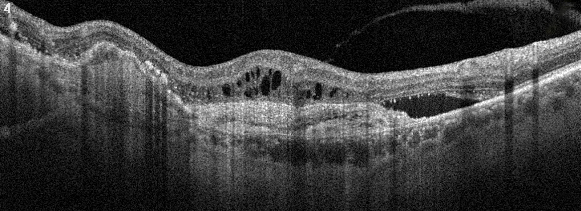

Right eye; optical coherence tomography B-scan.
Impression: AMD.